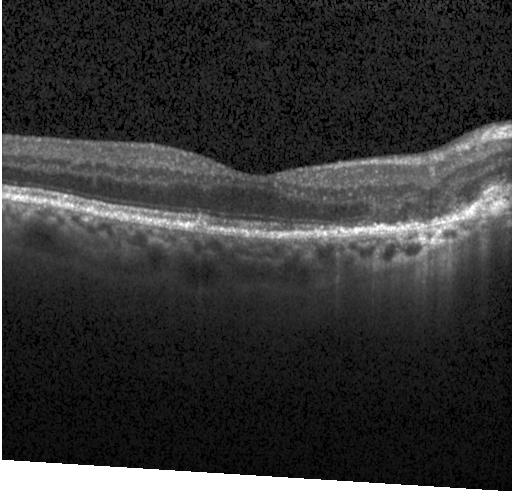
Spectral-domain OCT B-scan: CNV.